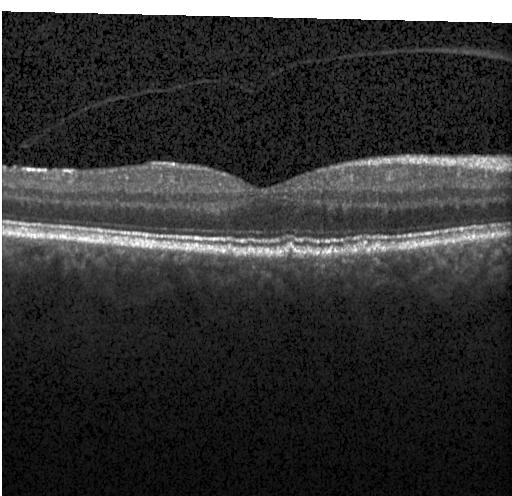

Diagnosis: sub-RPE drusenoid deposits.